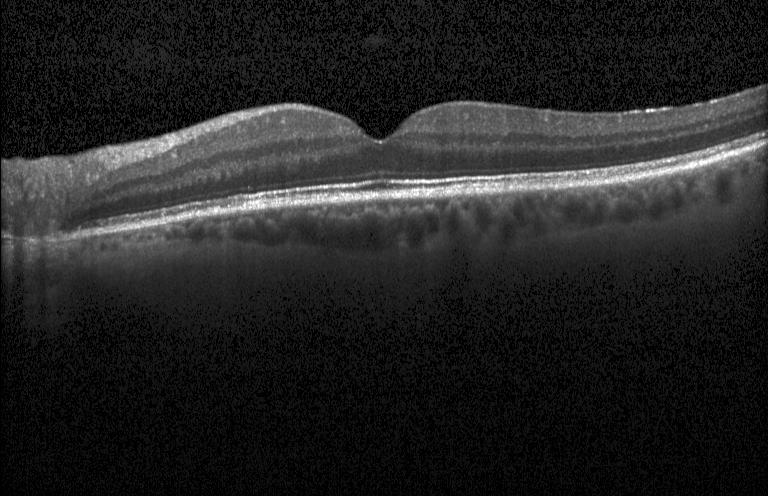
Diagnosis: no choroidal neovascularization, diabetic macular edema, or drusen.